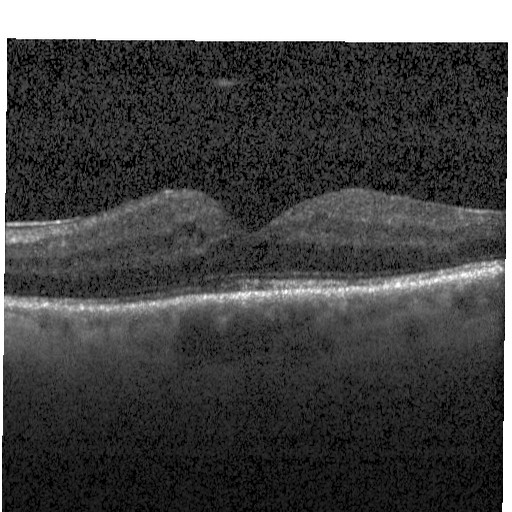 OCT B-scan. DME.